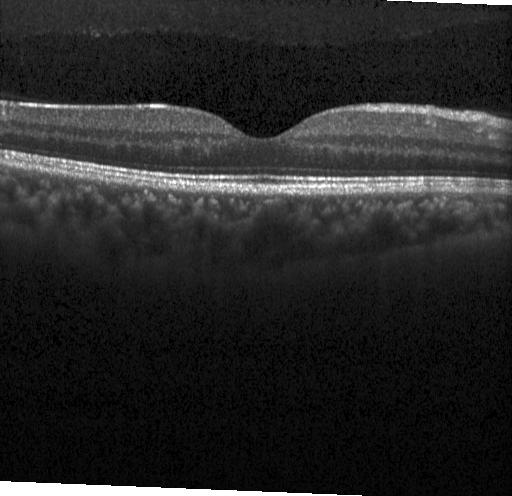

Optical coherence tomography B-scan; SD-OCT
Finding: neither choroidal neovascularization, diabetic macular edema, nor drusen.